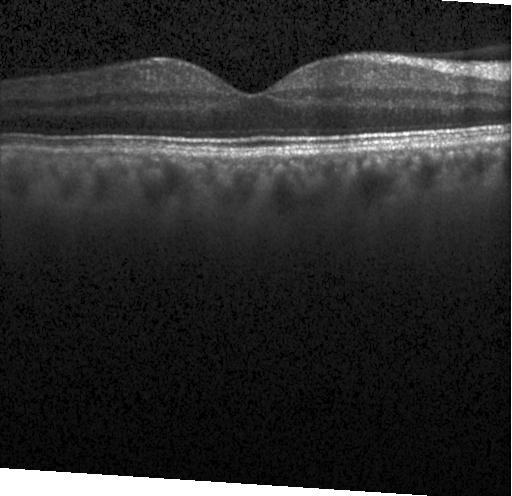 Spectral-domain OCT · horizontal scan through the fovea · instrument: Heidelberg Spectralis · optical coherence tomography scan — Impression: no CNV, DME, or drusen.